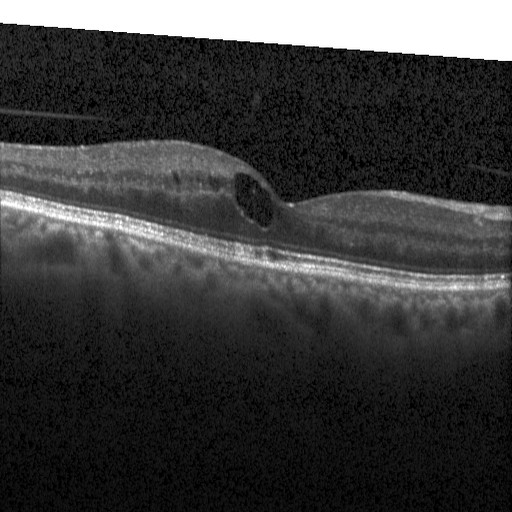
Horizontal scan through the fovea; Heidelberg Spectralis OCT system; spectral-domain optical coherence tomography; optical coherence tomography scan. Diabetic macular edema.